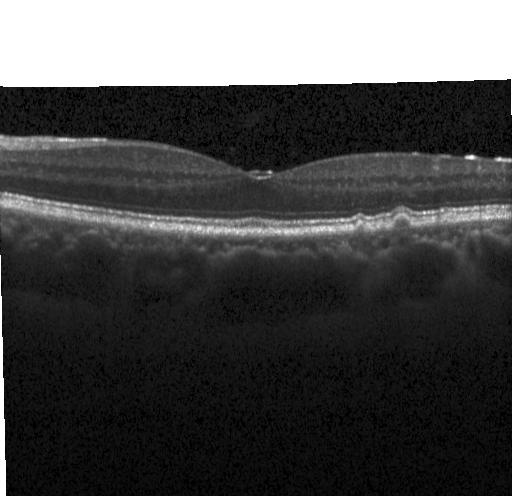

This B-scan demonstrates drusen.